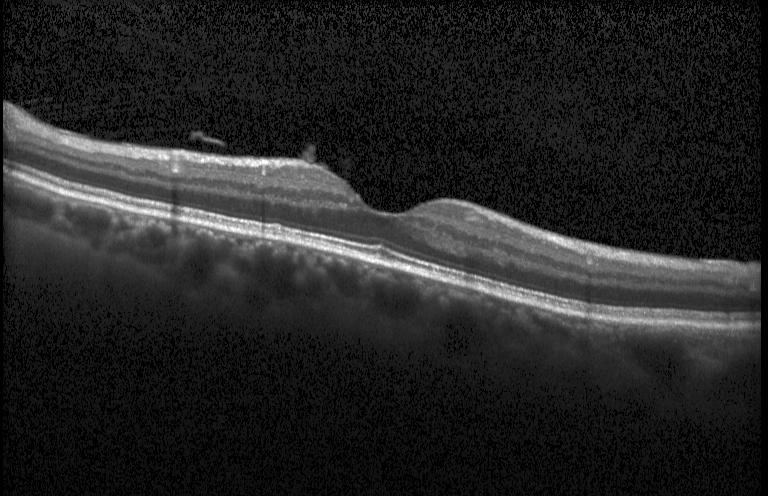
Assessment: no CNV, DME, or drusen.